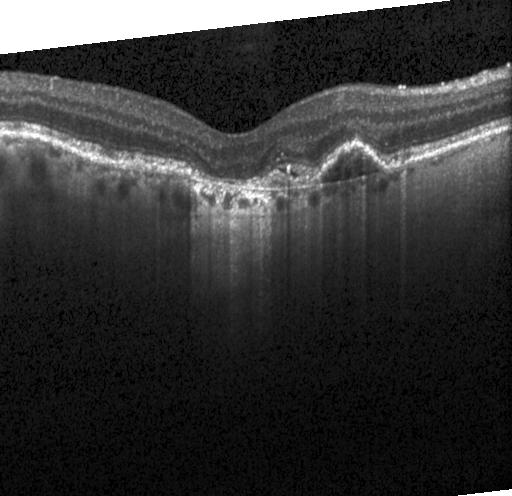
OCT finding: choroidal neovascularization.